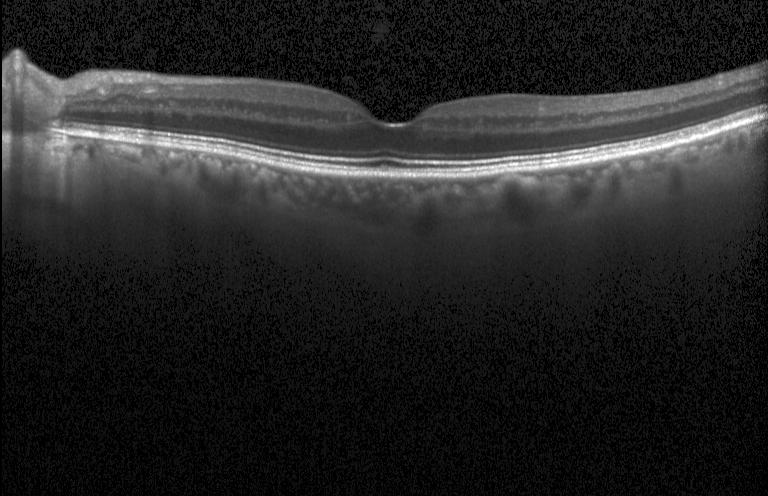

Spectral-domain OCT · Heidelberg Spectralis · OCT line scan. Diagnosis: no CNV, no DME, and no drusen.